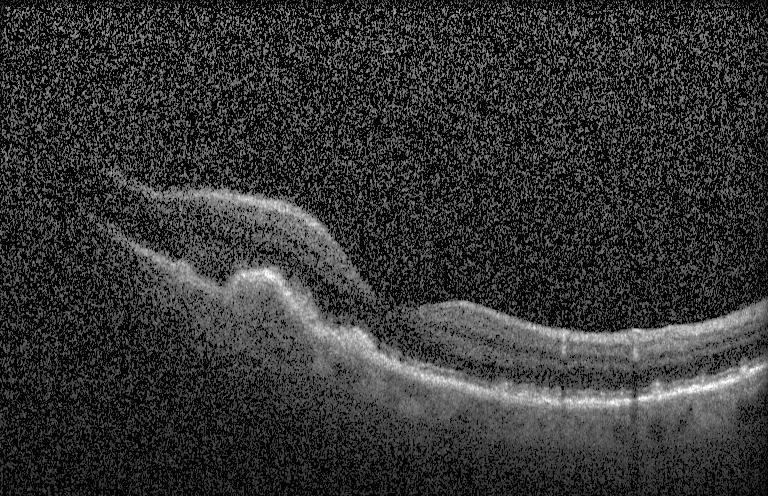

OCT B-scan showing a choroidal neovascular membrane.